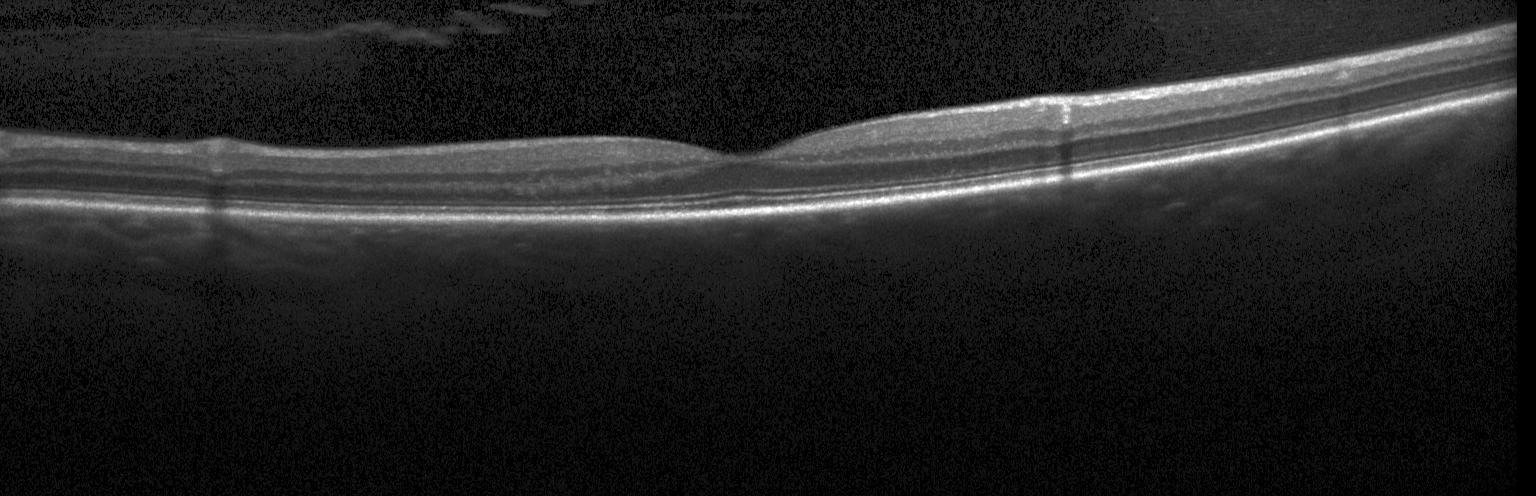 Spectral-domain OCT, fovea-centered, Heidelberg Spectralis OCT system, optical coherence tomography scan. Finding: no evidence of choroidal neovascularization, diabetic macular edema, or drusen.